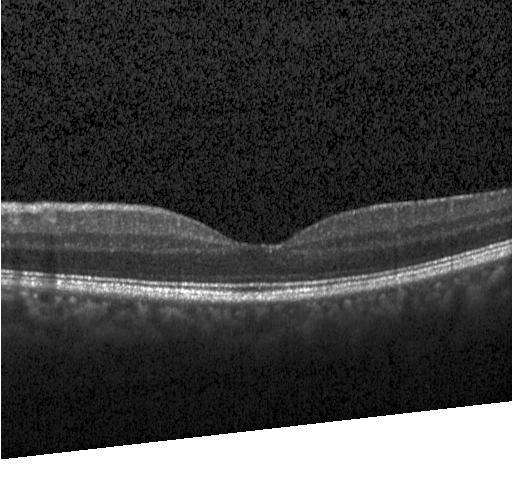
Acquired on a Heidelberg Spectralis, SD-OCT, macular scan, optical coherence tomography B-scan — Impression: no choroidal neovascularization, no diabetic macular edema, and no drusen.